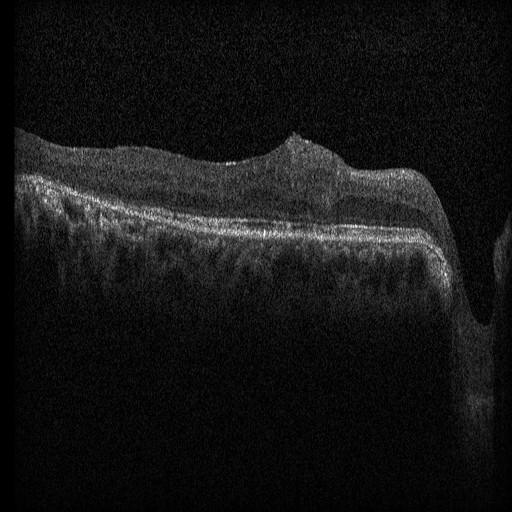

Retinal OCT B-scan, Heidelberg Spectralis OCT system. Diagnosis: diabetic macular edema.